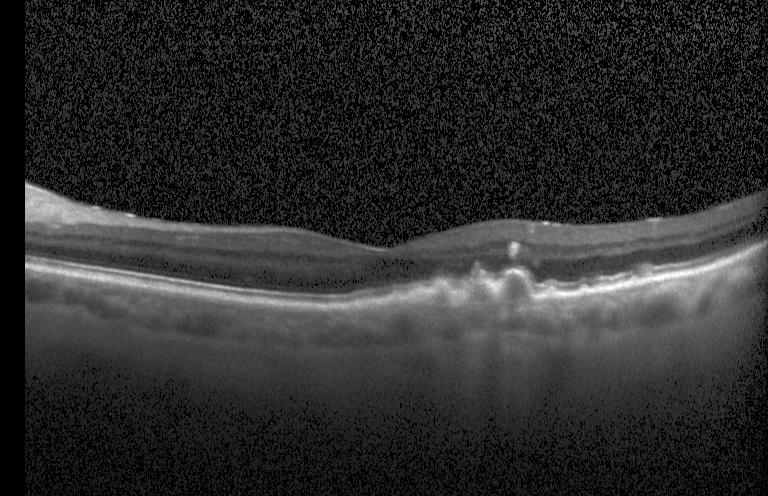 Dx: drusen.